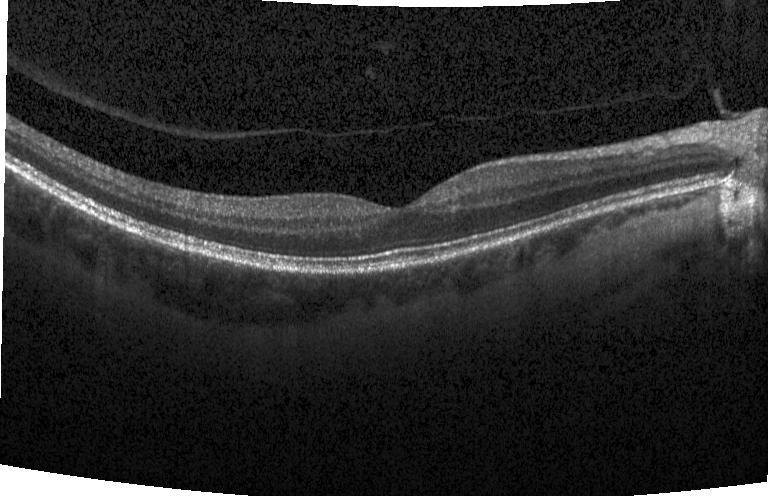 Macular OCT demonstrating no CNV, DME, or drusen.